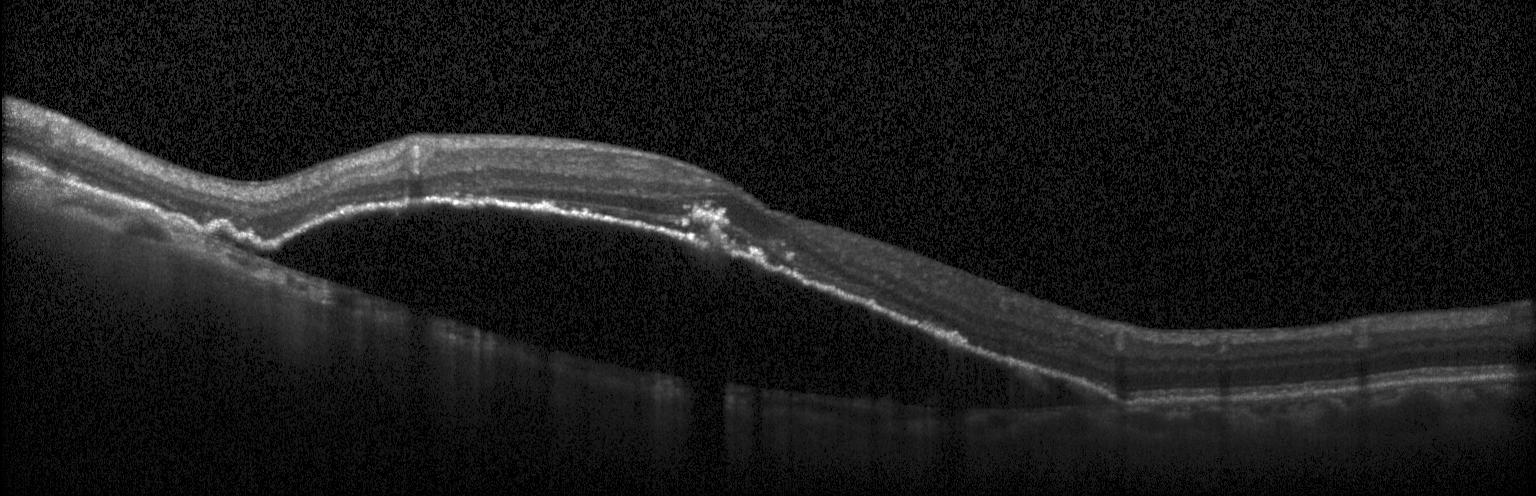

OCT B-scan; horizontal scan through the fovea; Heidelberg Spectralis.
Diagnosis: a choroidal neovascular membrane.